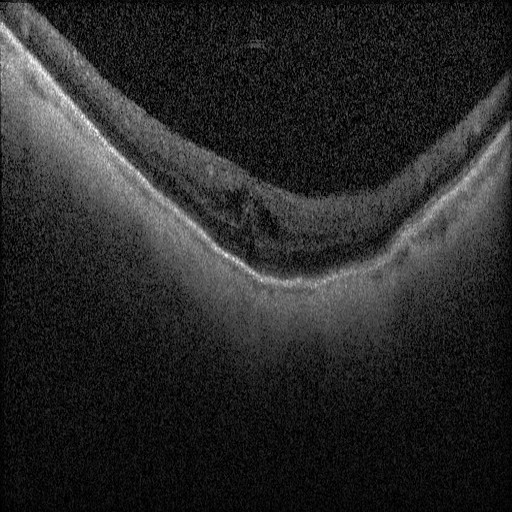 Macular OCT: diabetic macular edema (DME).